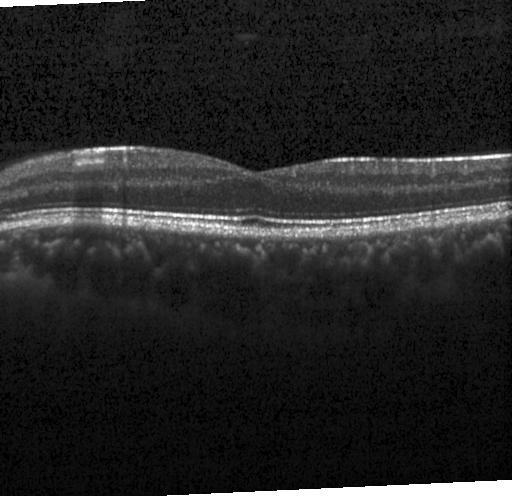

Retinal OCT cross-section showing no choroidal neovascularization, diabetic macular edema, or drusen.